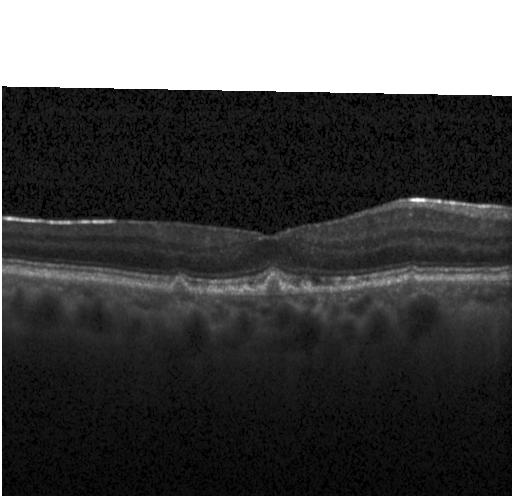

Optical coherence tomography B-scan, SD-OCT, Heidelberg Spectralis. Finding: drusen.